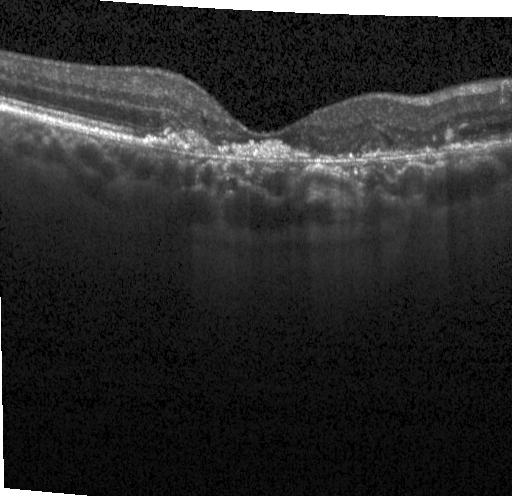
Assessment: choroidal neovascularization.